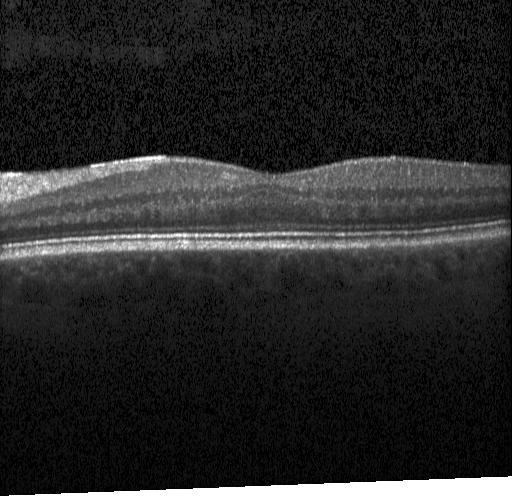

Spectral-domain optical coherence tomography. Retinal OCT cross-section.
OCT finding: no choroidal neovascularization, diabetic macular edema, or drusen.